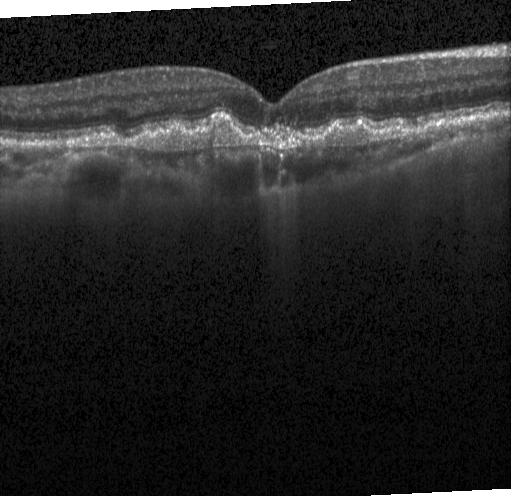

Retinal OCT cross-section showing a choroidal neovascular membrane.